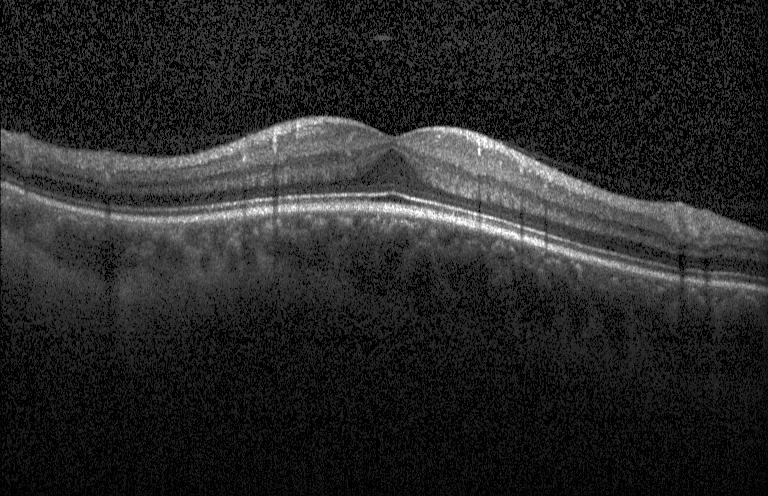
Spectral-domain optical coherence tomography, OCT line scan.
Diagnosis: no choroidal neovascularization, diabetic macular edema, or drusen.